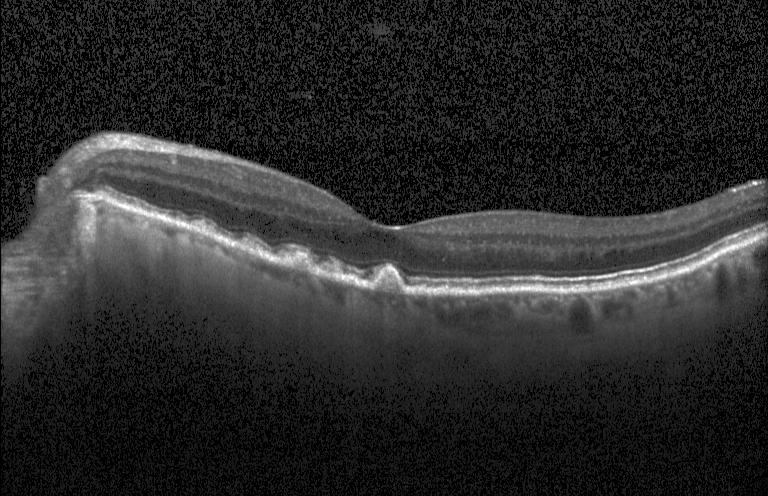
Spectral-domain OCT B-scan: multiple drusen.